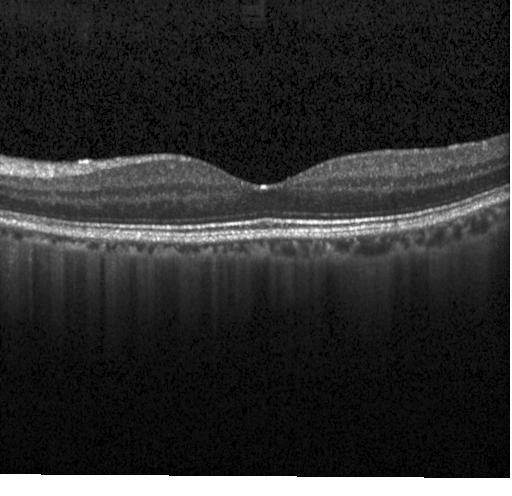

Macular OCT: no choroidal neovascularization, diabetic macular edema, or drusen.